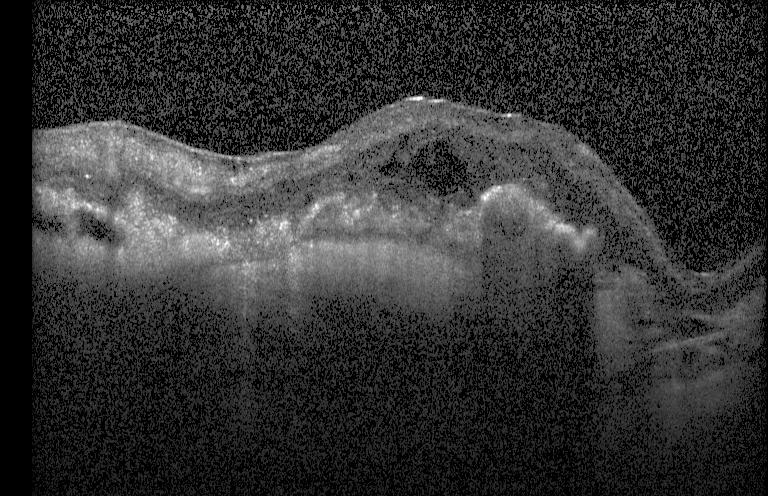
Spectral-domain optical coherence tomography. OCT B-scan. Horizontal scan through the fovea. Finding: choroidal neovascularization (CNV).